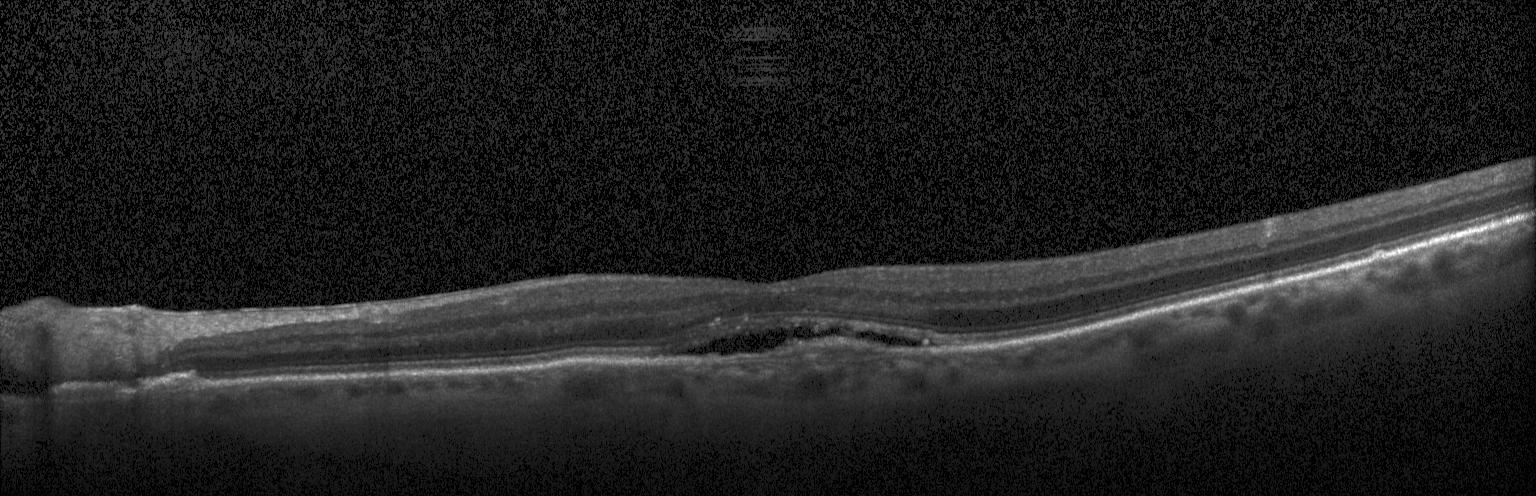
Heidelberg Spectralis. OCT line scan. Fovea-centered. SD-OCT — Assessment: CNV.